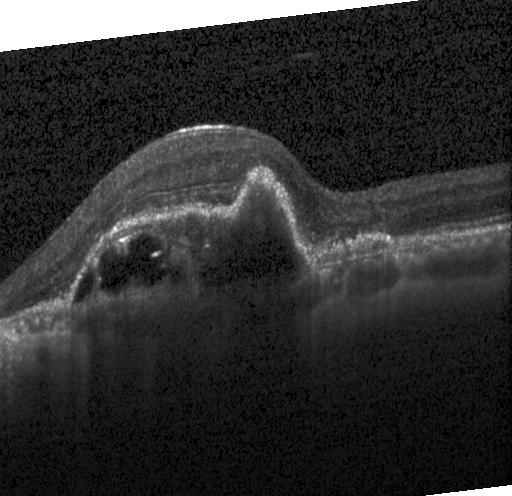
SD-OCT, optical coherence tomography B-scan, acquired on a Heidelberg Spectralis — Macular OCT: CNV.